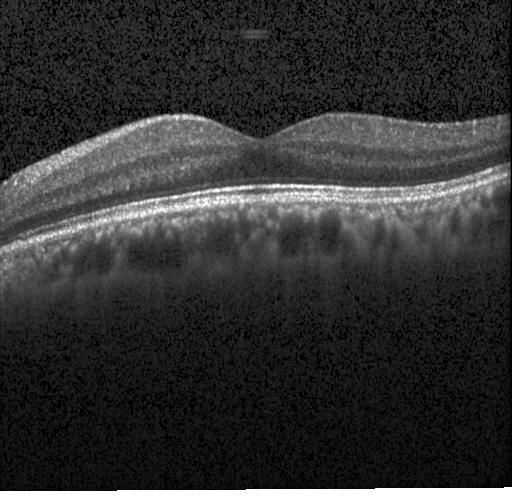 Horizontal scan through the fovea; optical coherence tomography B-scan — Impression: no evidence of choroidal neovascularization, diabetic macular edema, or drusen.